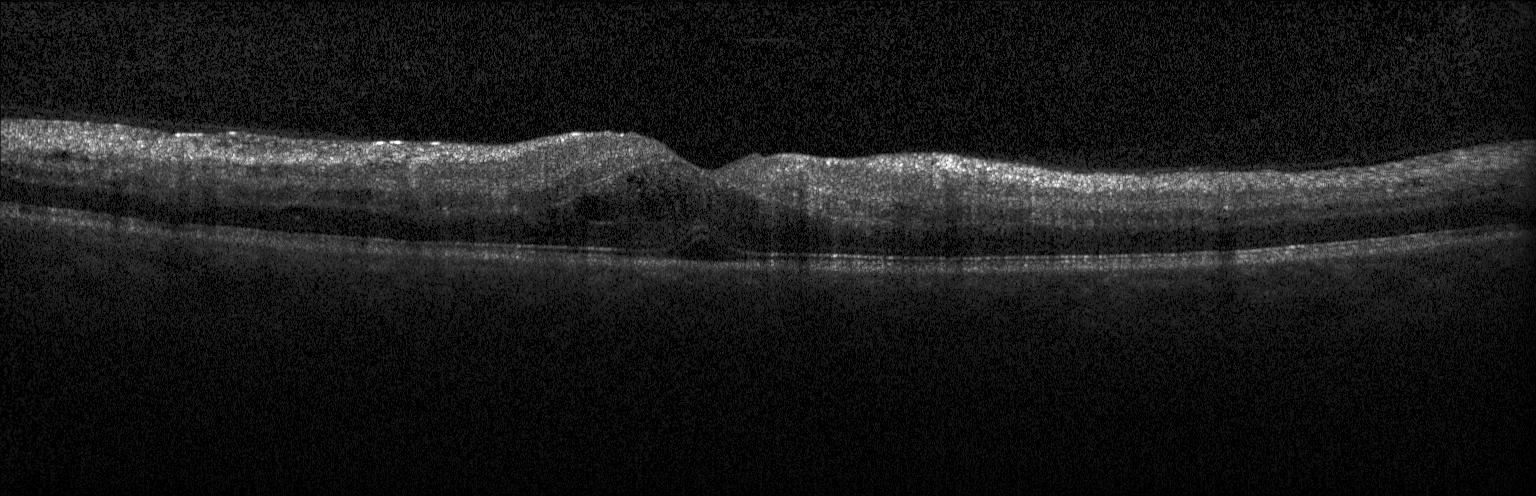 Spectral-domain optical coherence tomography. Optical coherence tomography scan
Diabetic macular edema (DME).